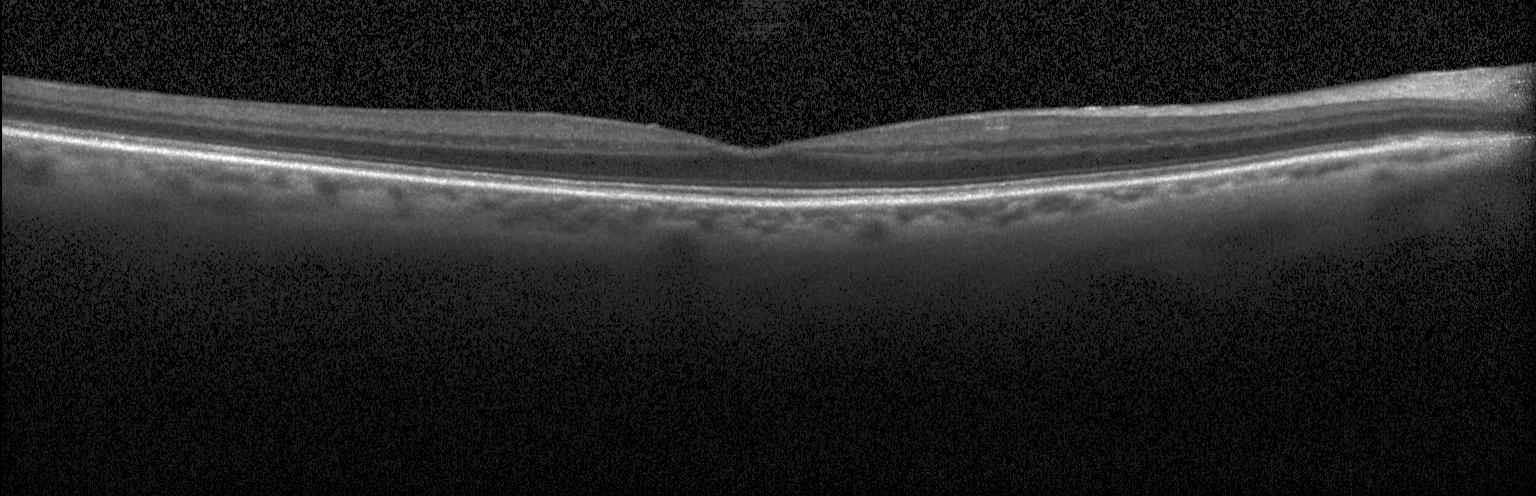
OCT scan showing no CNV, no DME, and no drusen.